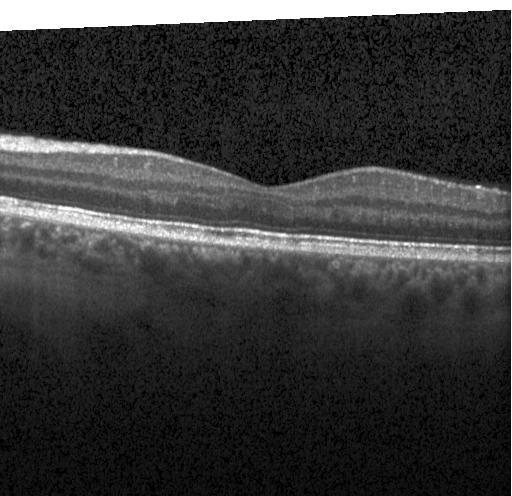 Impression: no evidence of choroidal neovascularization, diabetic macular edema, or drusen.